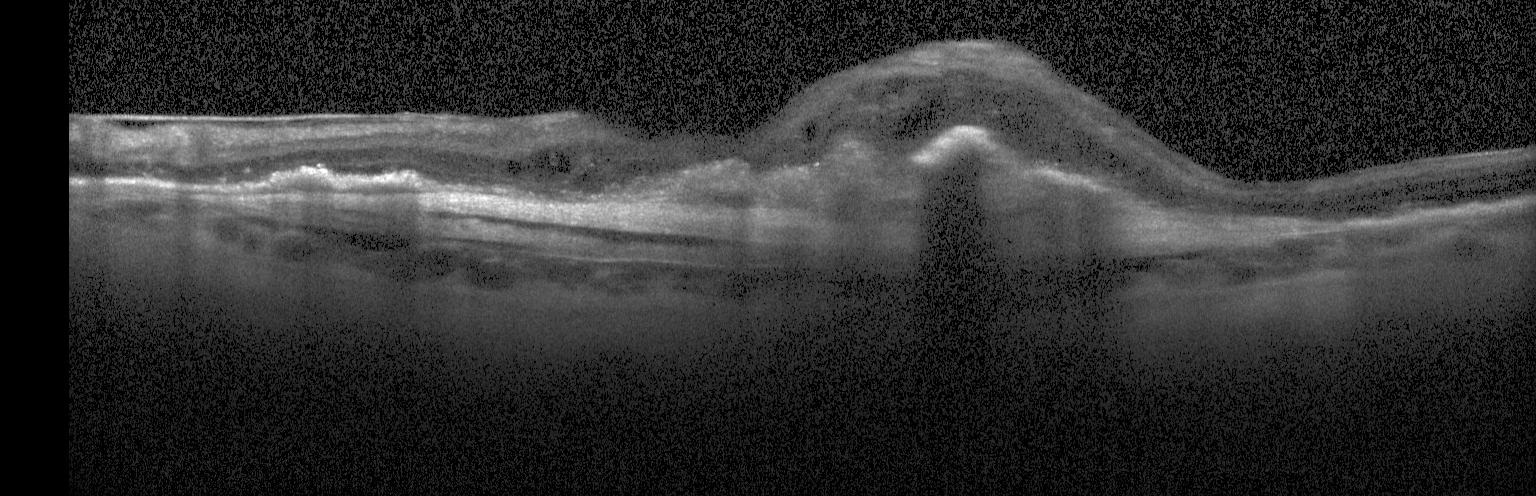
OCT B-scan. Impression: CNV.